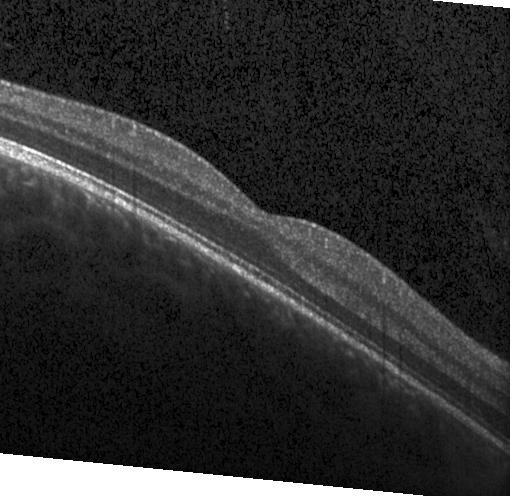 Macular scan · OCT line scan · spectral-domain OCT.
Dx: no choroidal neovascularization, no diabetic macular edema, and no drusen.